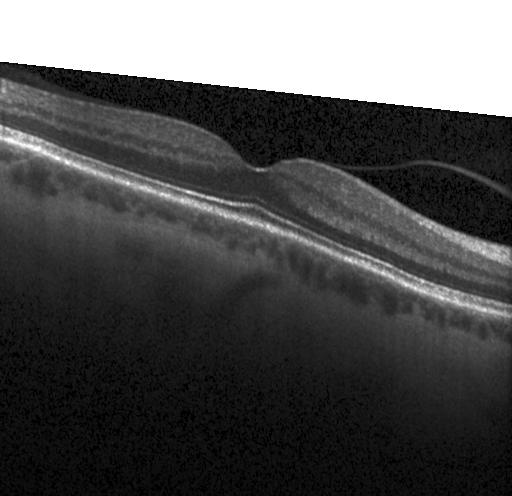 Optical coherence tomography B-scan, SD-OCT — Finding: no evidence of CNV, DME, or drusen.